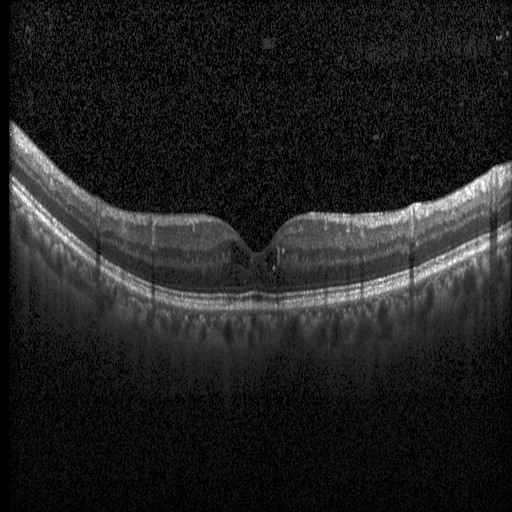 Spectral-domain OCT B-scan: diabetic macular edema.